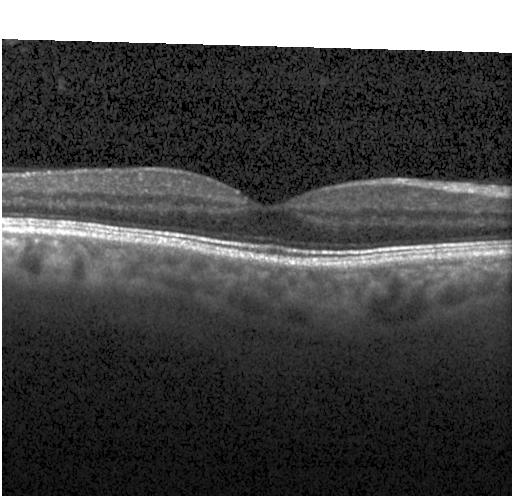

Impression: no choroidal neovascularization, no diabetic macular edema, and no drusen.